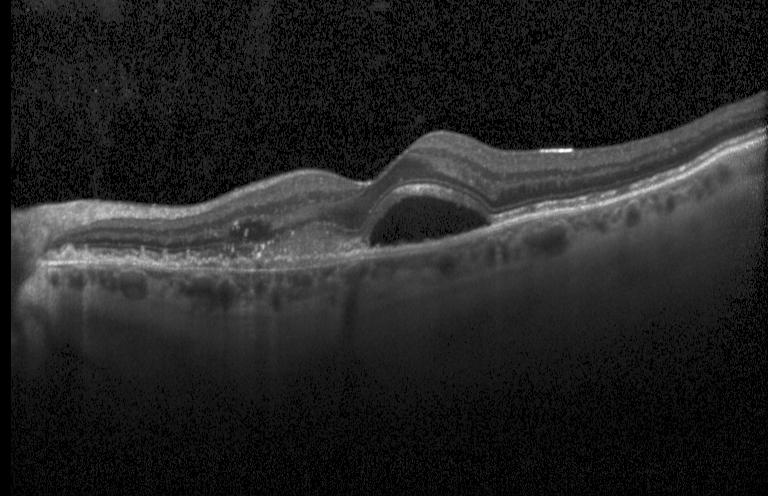

OCT line scan; SD-OCT; acquired on a Heidelberg Spectralis; centered on the fovea — OCT finding: a choroidal neovascular membrane.